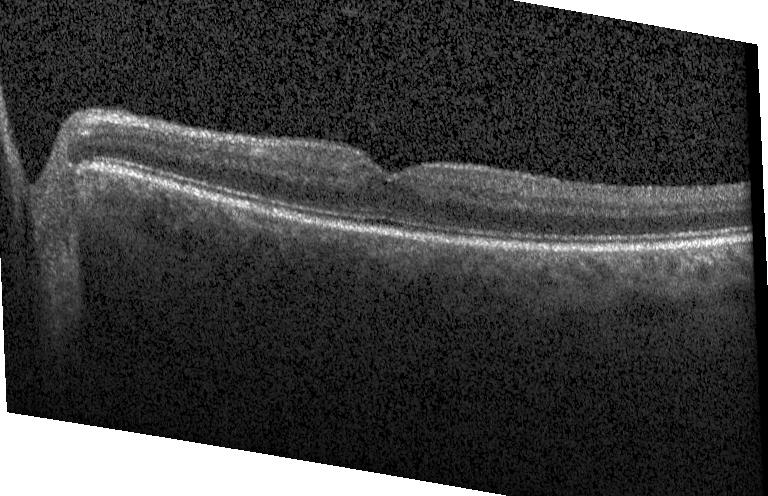
Retinal OCT B-scan · horizontal scan through the fovea · Heidelberg Spectralis OCT system · spectral-domain optical coherence tomography. OCT finding: no CNV, no DME, and no drusen.